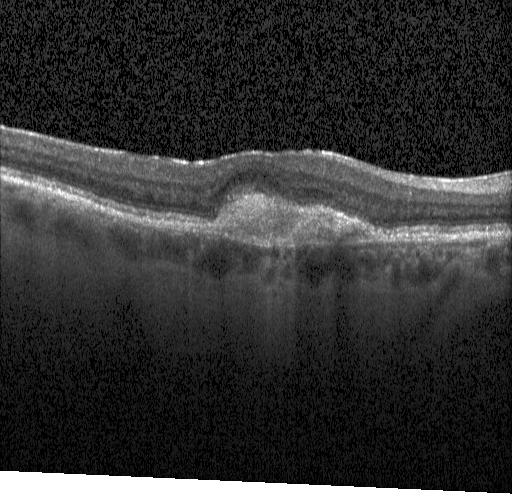

SD-OCT · through the macula · optical coherence tomography scan · Heidelberg Spectralis OCT system. Finding: CNV.